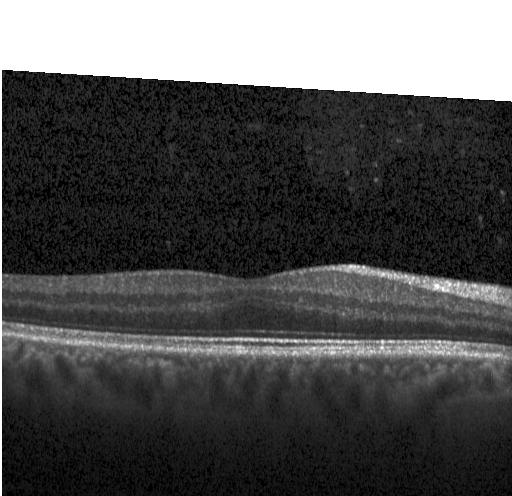
Instrument: Heidelberg Spectralis; centered on the fovea; OCT B-scan; SD-OCT. Impression: neither CNV, DME, nor drusen.